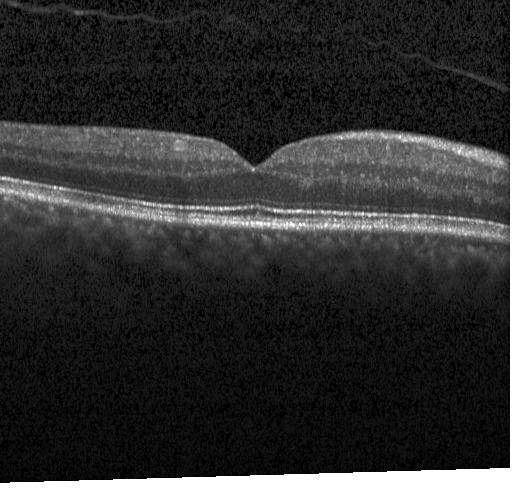
Optical coherence tomography scan.
OCT finding: no evidence of choroidal neovascularization, diabetic macular edema, or drusen.